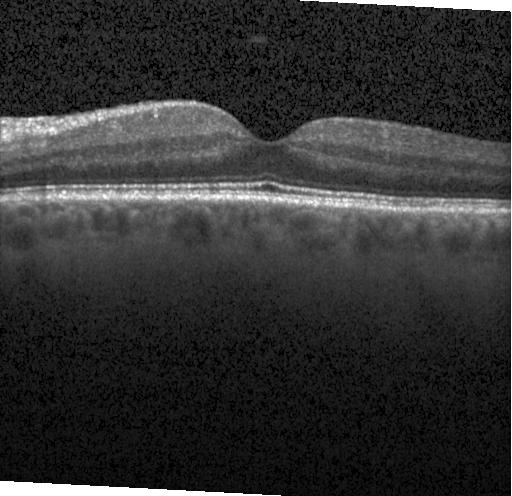
Through the macula, optical coherence tomography B-scan
Impression: no CNV, DME, or drusen.